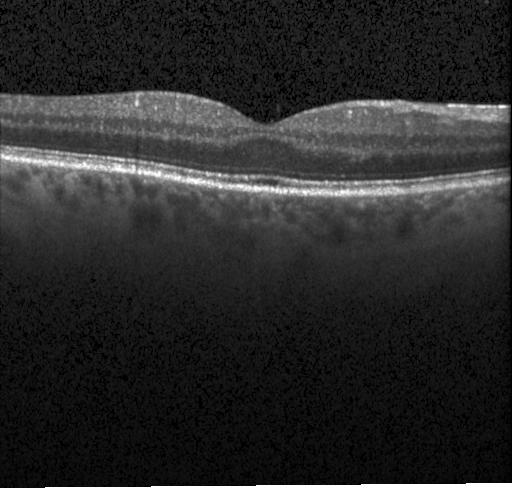
Heidelberg Spectralis OCT system. Retinal OCT B-scan. Impression: no choroidal neovascularization, no diabetic macular edema, and no drusen.